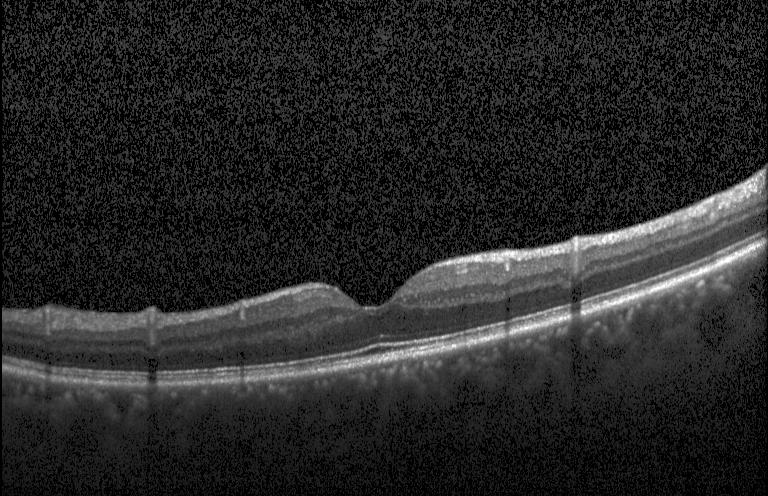

Optical coherence tomography B-scan, through the macula.
Finding: no evidence of CNV, DME, or drusen.